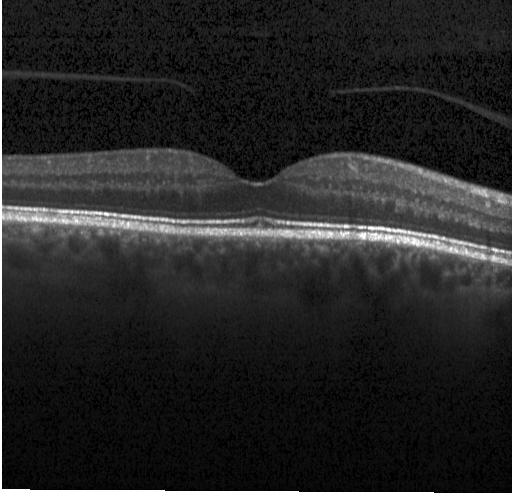
OCT finding: neither CNV, DME, nor drusen.